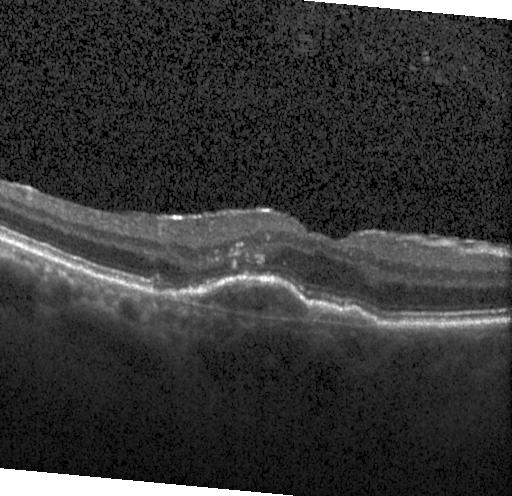 Macular OCT: a choroidal neovascular membrane.